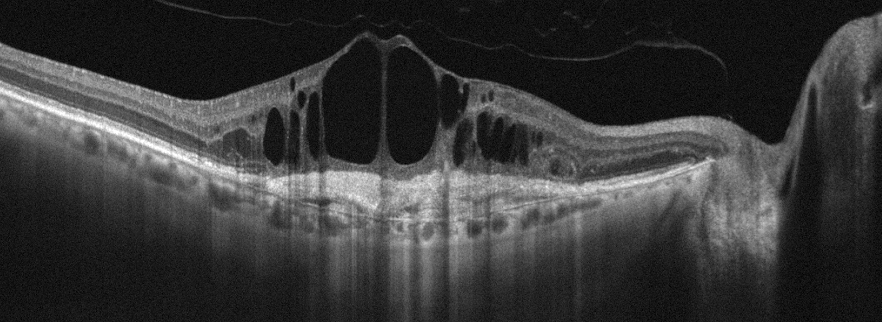

Macular scan; retinal OCT B-scan; right eye; instrument: Optovue Avanti RTVue XR. This B-scan demonstrates age-related macular degeneration (AMD).